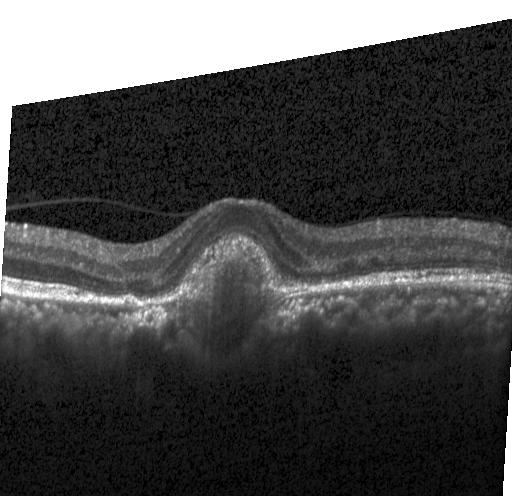
OCT line scan
A choroidal neovascular membrane.